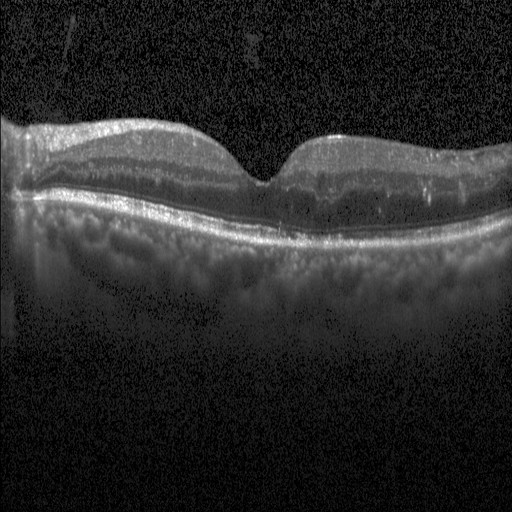
Spectral-domain OCT; optical coherence tomography B-scan; horizontal scan through the fovea
Diabetic macular edema (DME).